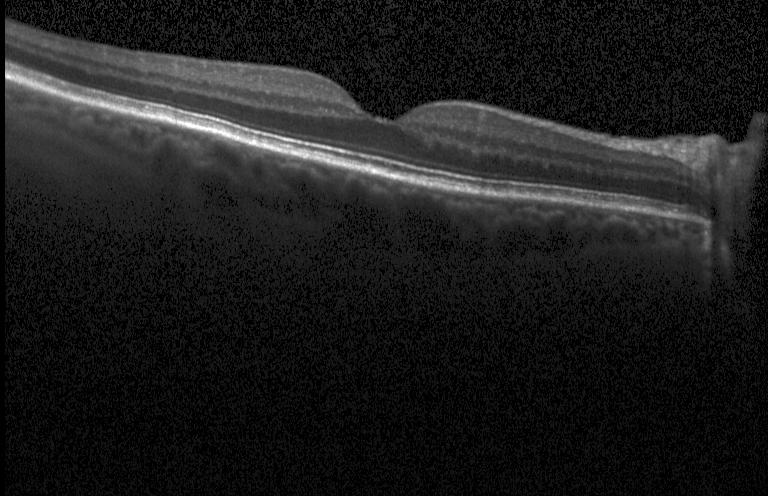
Instrument: Heidelberg Spectralis; horizontal scan through the fovea; retinal OCT B-scan.
Assessment: no evidence of choroidal neovascularization, diabetic macular edema, or drusen.